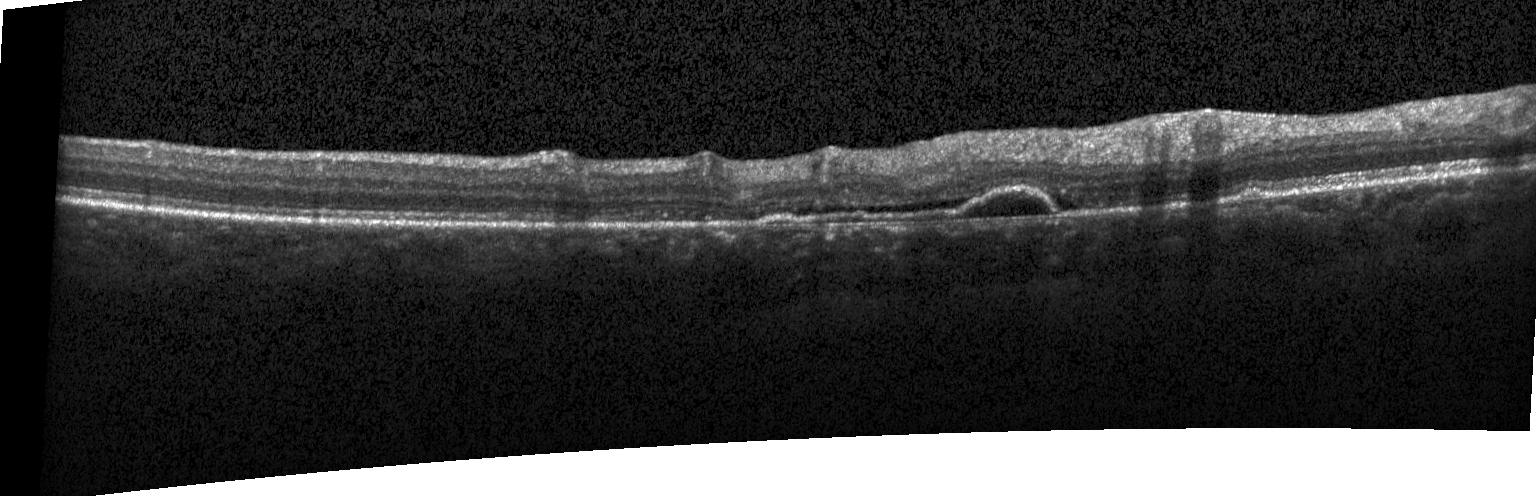 A choroidal neovascular membrane.